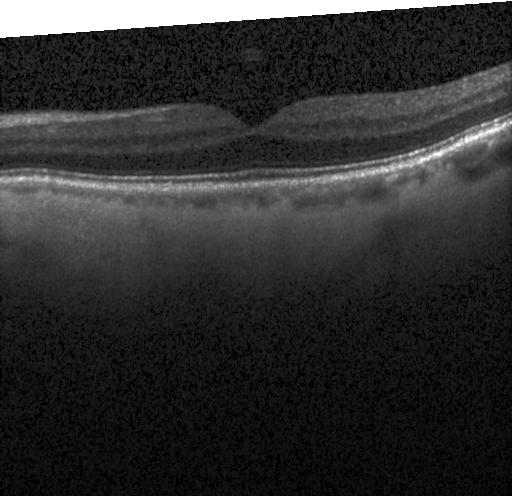 OCT line scan.
Finding: no evidence of CNV, DME, or drusen.